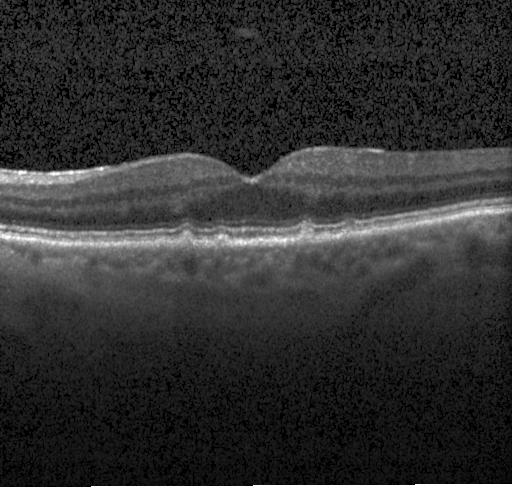

Acquired on a Heidelberg Spectralis, optical coherence tomography B-scan, spectral-domain OCT. Impression: multiple drusen.